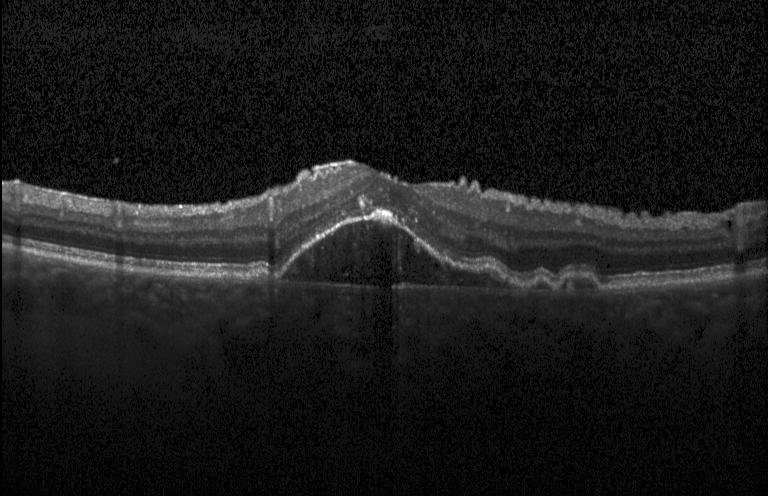
Optical coherence tomography B-scan.
Finding: choroidal neovascularization.